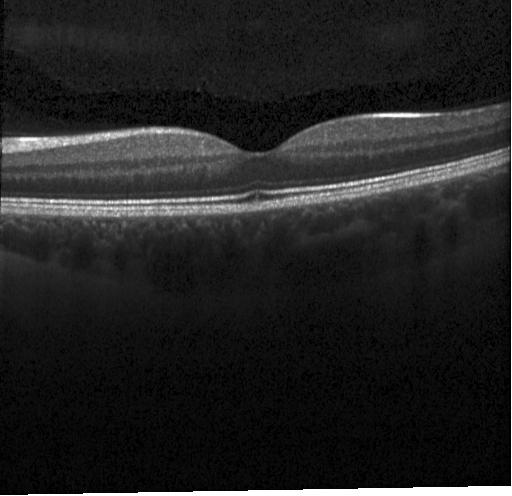

Retinal OCT B-scan. Impression: no choroidal neovascularization, no diabetic macular edema, and no drusen.